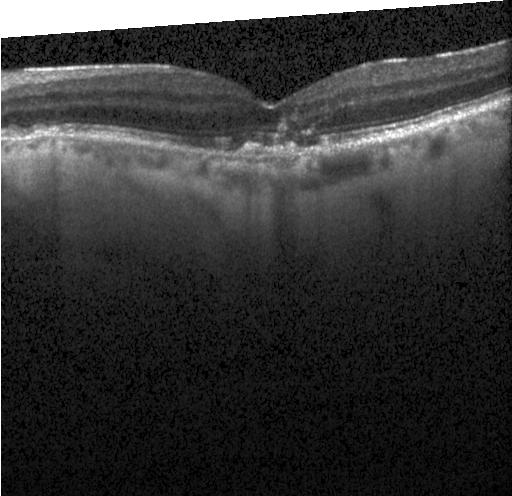
Spectral-domain optical coherence tomography, OCT B-scan
Diagnosis: CNV.